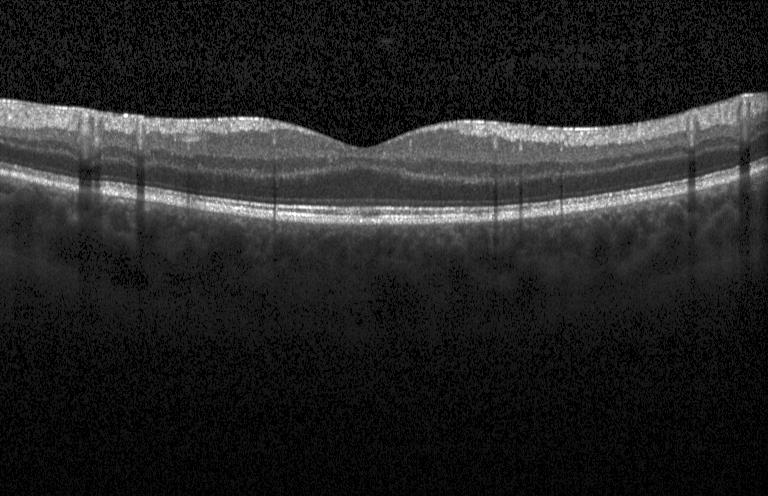 Spectral-domain optical coherence tomography, optical coherence tomography scan, instrument: Heidelberg Spectralis. Finding: neither choroidal neovascularization, diabetic macular edema, nor drusen.